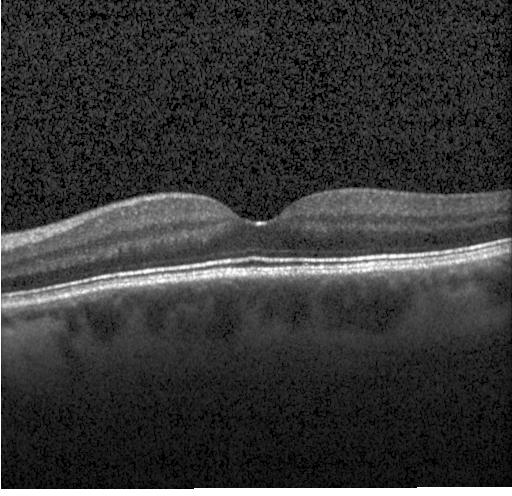

OCT finding: no choroidal neovascularization, no diabetic macular edema, and no drusen.